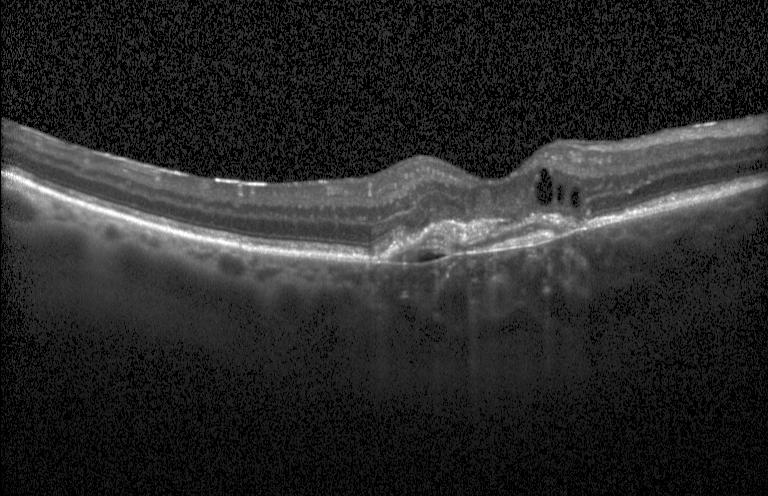

Finding: choroidal neovascularization (CNV).